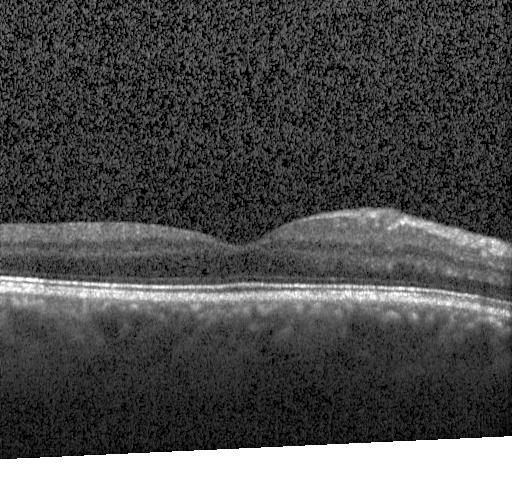

Retinal OCT cross-section; macular scan
No choroidal neovascularization, diabetic macular edema, or drusen.